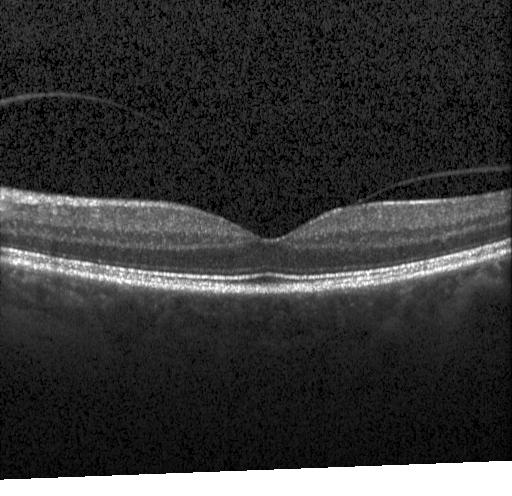
Centered on the fovea, retinal OCT cross-section, instrument: Heidelberg Spectralis. Impression: no CNV, DME, or drusen.